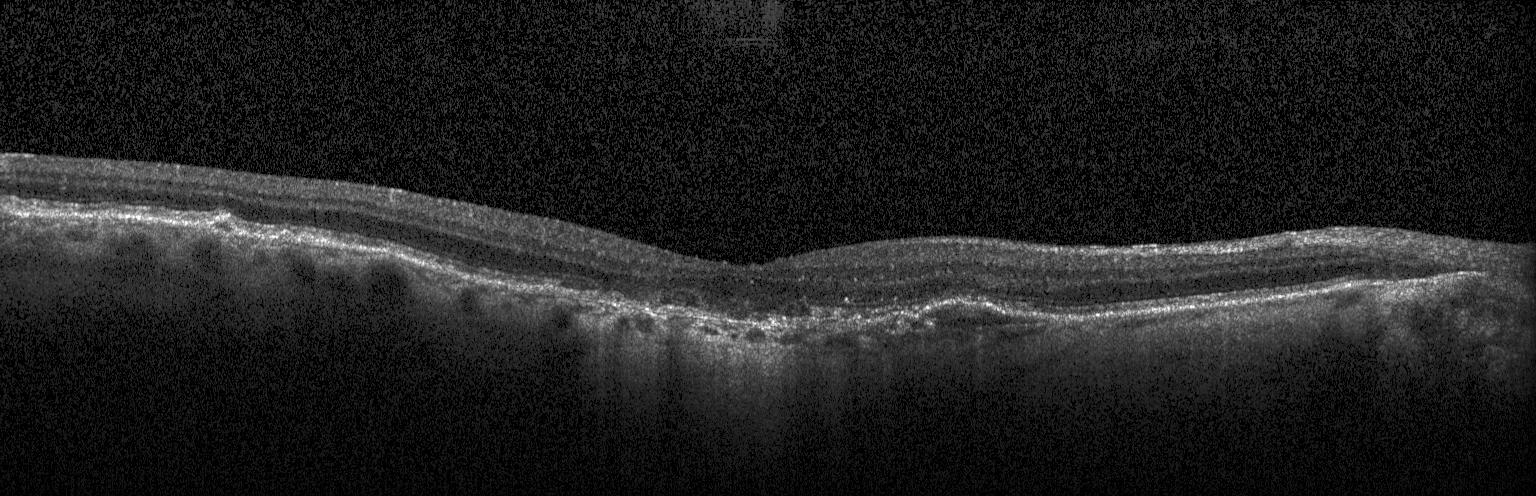

Optical coherence tomography B-scan.
Assessment: CNV.